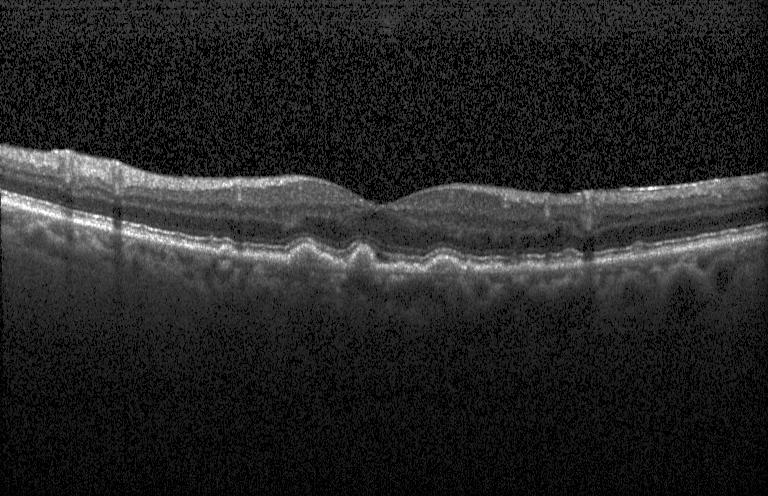

Optical coherence tomography B-scan; through the macula; acquired on a Heidelberg Spectralis.
OCT finding: multiple drusen.